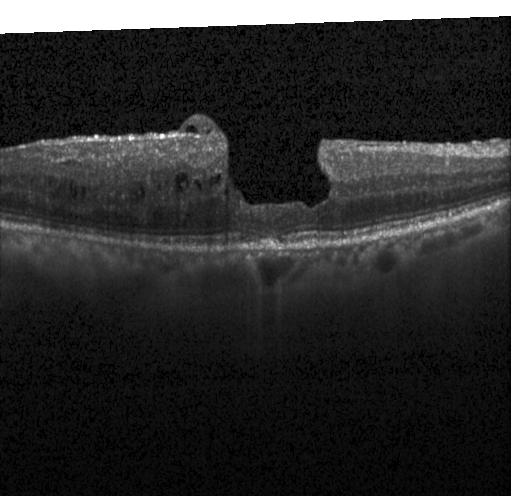

Finding: diabetic macular edema.